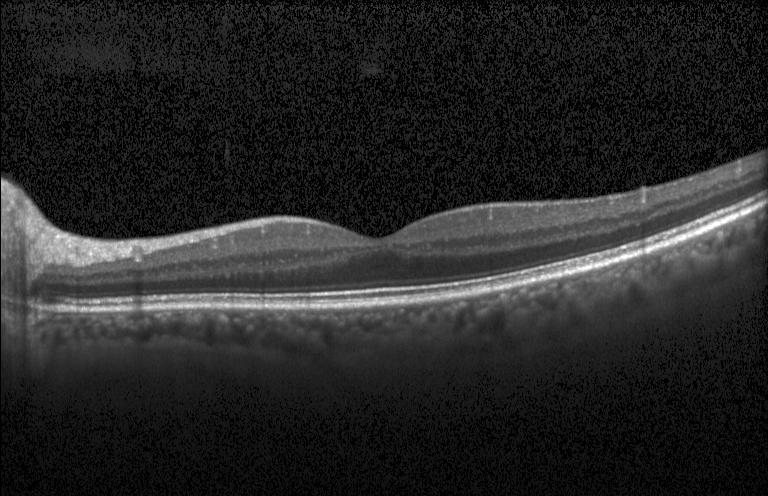
Retinal OCT B-scan.
Assessment: no choroidal neovascularization, diabetic macular edema, or drusen.